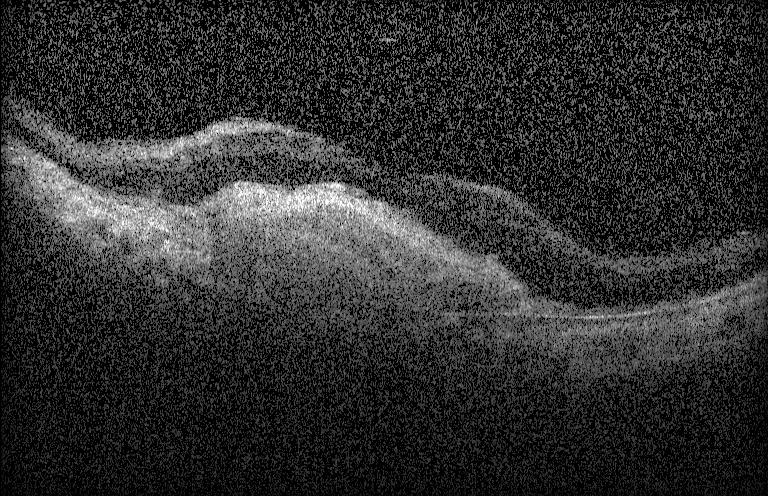
Retinal OCT cross-section. Assessment: a choroidal neovascular membrane.